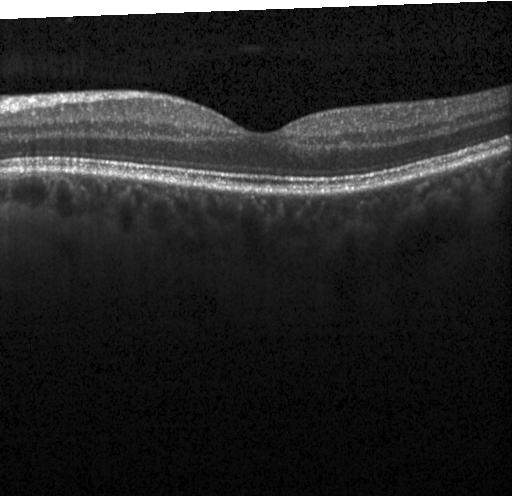

Fovea-centered. Instrument: Heidelberg Spectralis. Spectral-domain optical coherence tomography. Retinal OCT B-scan.
OCT finding: no evidence of choroidal neovascularization, diabetic macular edema, or drusen.